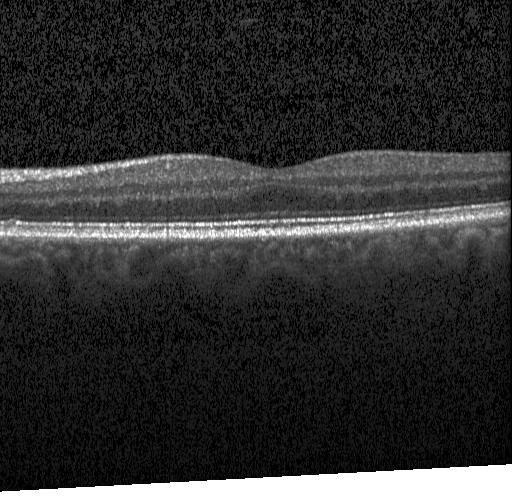
Optical coherence tomography scan · fovea-centered — Assessment: neither choroidal neovascularization, diabetic macular edema, nor drusen.